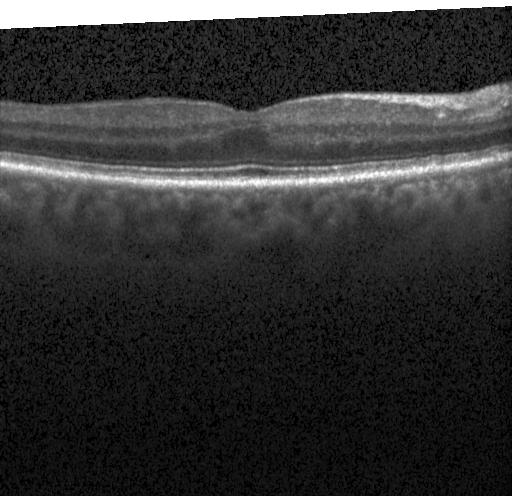

OCT B-scan. Diagnosis: no evidence of choroidal neovascularization, diabetic macular edema, or drusen.